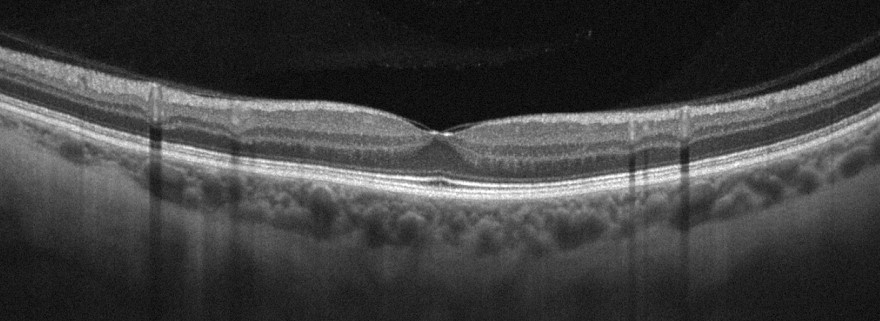 Optical coherence tomography scan — Diagnosis: absence of AMD, DME, ERM, RAO, RVO, and vitreomacular interface disease.